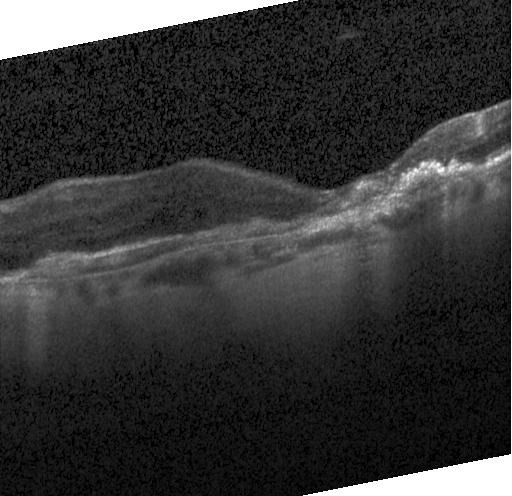

Finding: choroidal neovascularization.